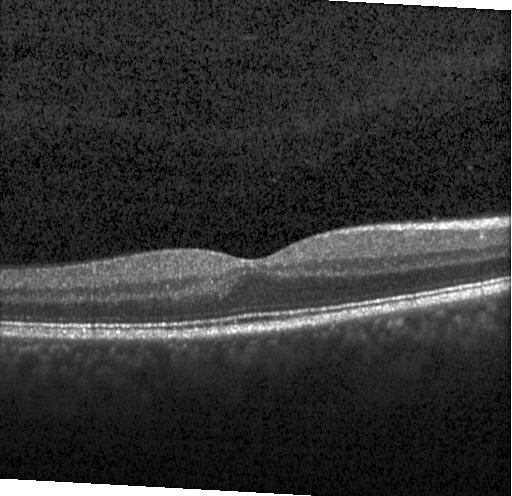
Impression: no evidence of choroidal neovascularization, diabetic macular edema, or drusen.